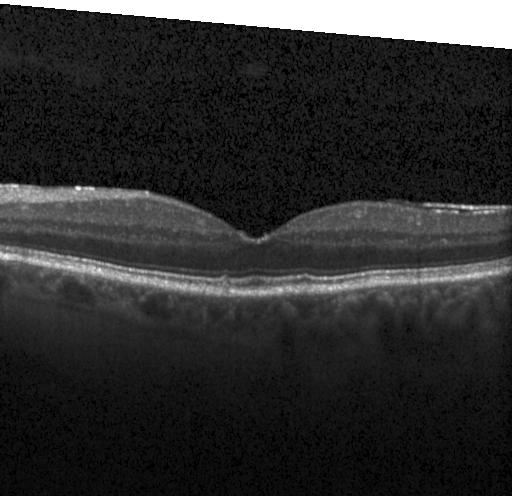
OCT line scan, acquired on a Heidelberg Spectralis. OCT finding: multiple drusen.